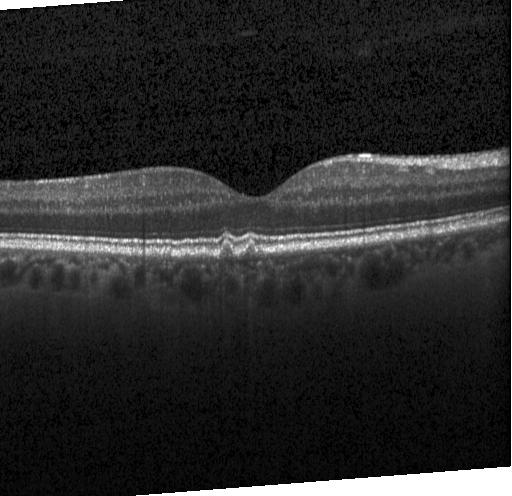
Dx: sub-RPE drusenoid deposits.